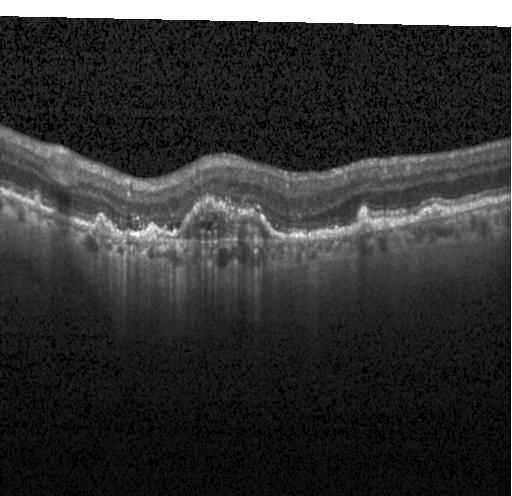 Diagnosis: a choroidal neovascular membrane.